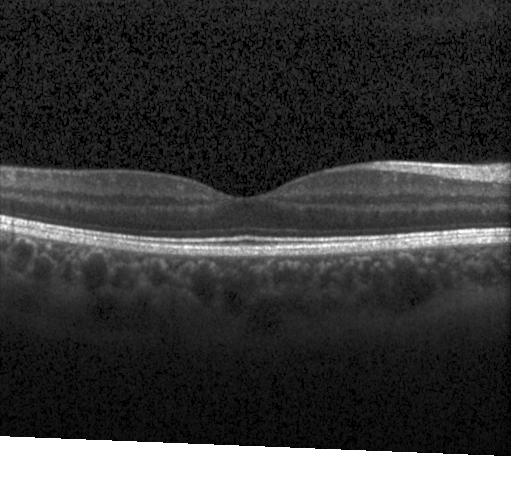

OCT B-scan — Impression: no evidence of CNV, DME, or drusen.